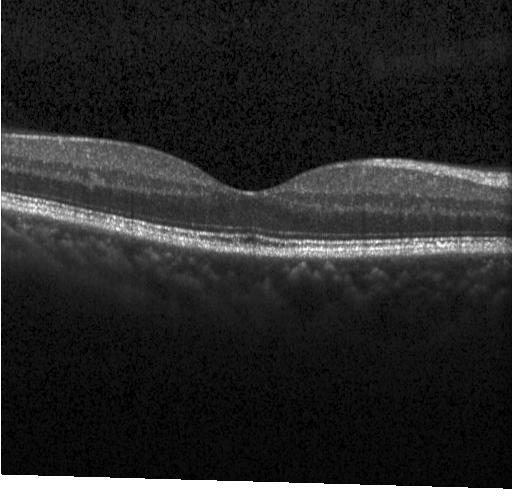

Through the macula; SD-OCT; acquired on a Heidelberg Spectralis; retinal OCT cross-section — Impression: no evidence of choroidal neovascularization, diabetic macular edema, or drusen.